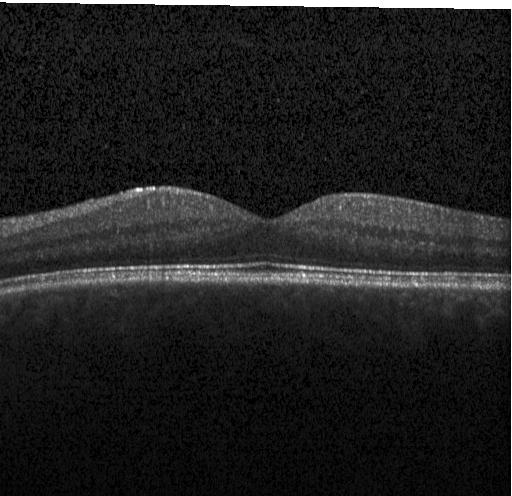

Fovea-centered. Optical coherence tomography scan. SD-OCT. Heidelberg Spectralis OCT system.
No CNV, no DME, and no drusen.